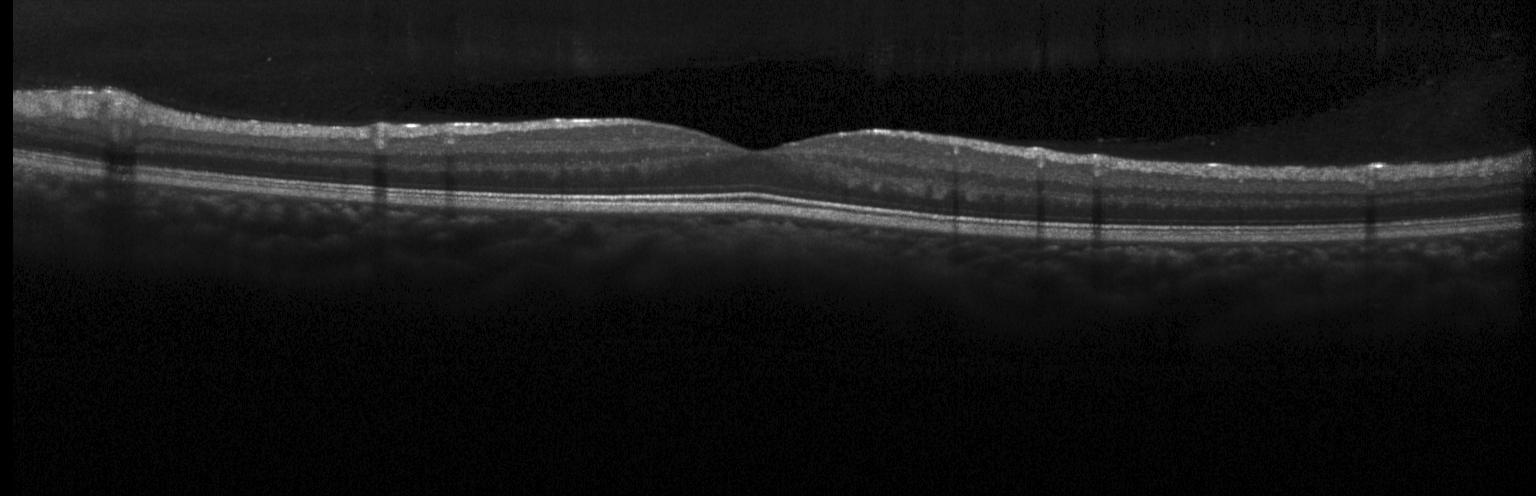
Retinal OCT cross-section, horizontal scan through the fovea — Finding: no CNV, no DME, and no drusen.